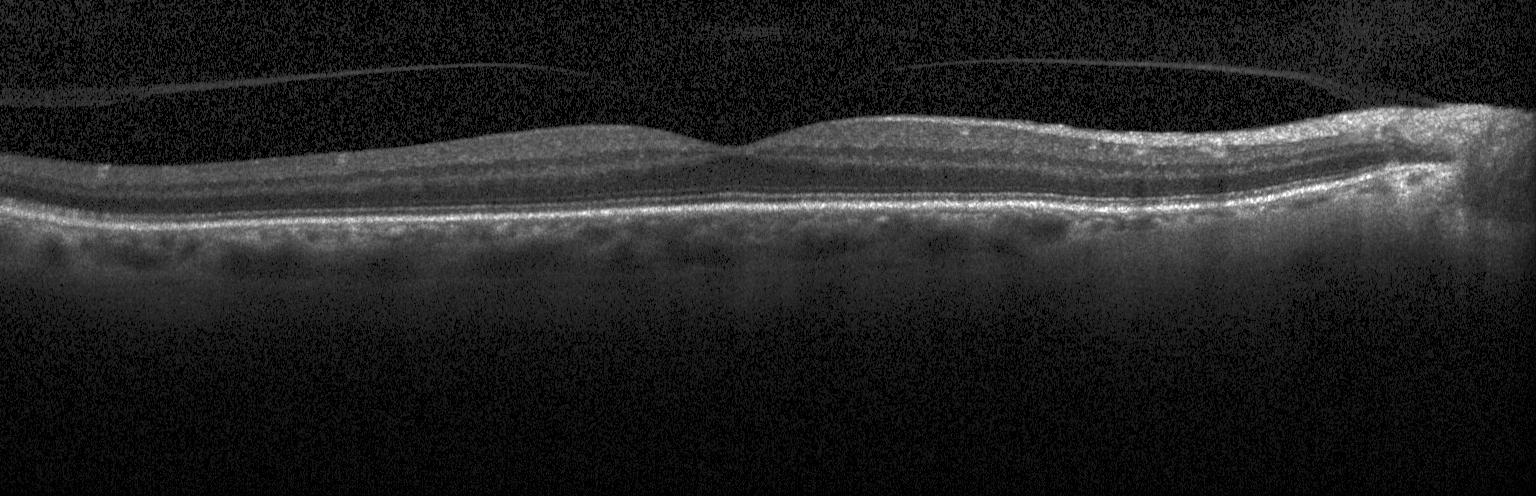
Retinal OCT cross-section; spectral-domain optical coherence tomography. Assessment: no choroidal neovascularization, diabetic macular edema, or drusen.